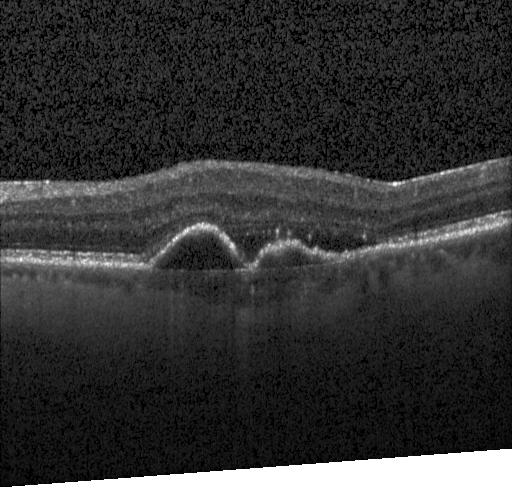
Optical coherence tomography B-scan — This B-scan demonstrates CNV.